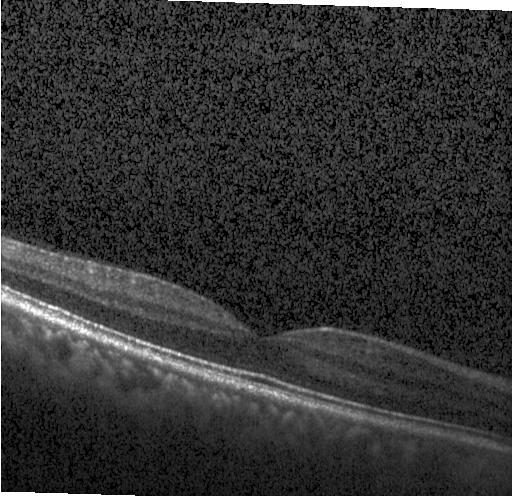
Diagnosis: neither choroidal neovascularization, diabetic macular edema, nor drusen.